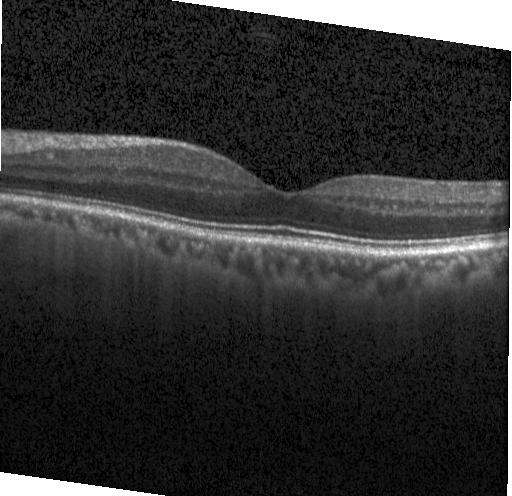 No choroidal neovascularization, diabetic macular edema, or drusen.